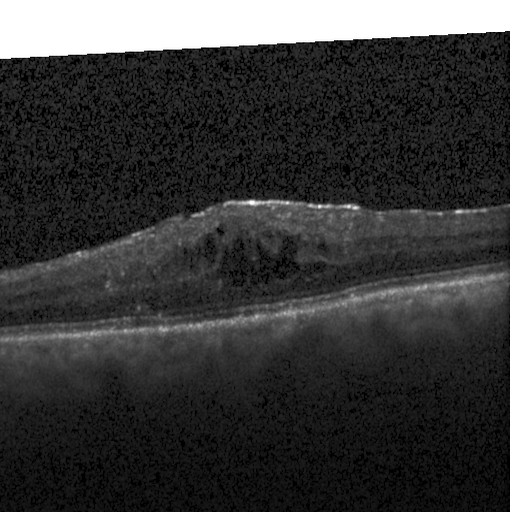

Dx: diabetic macular edema (DME).